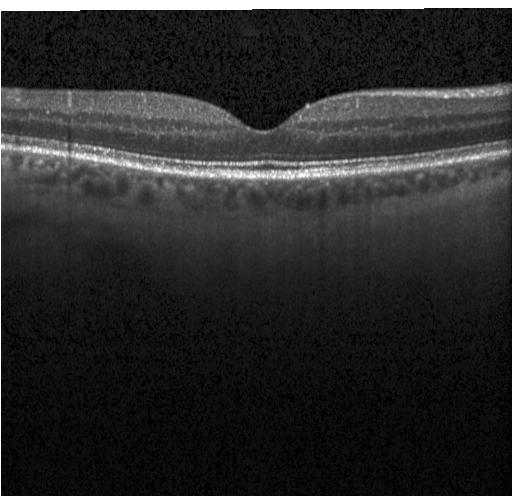 SD-OCT, retinal OCT B-scan, Heidelberg Spectralis.
Finding: no choroidal neovascularization, no diabetic macular edema, and no drusen.